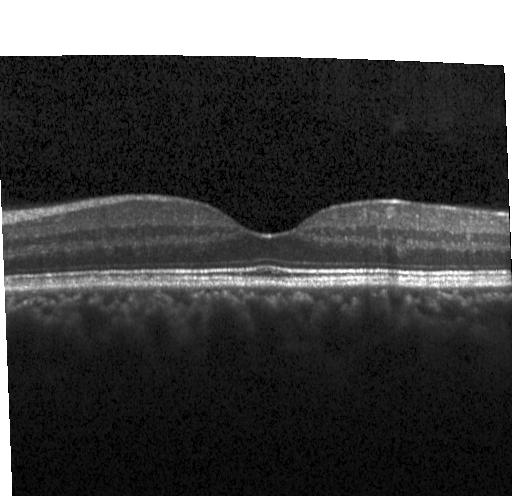 Impression: no choroidal neovascularization, diabetic macular edema, or drusen.